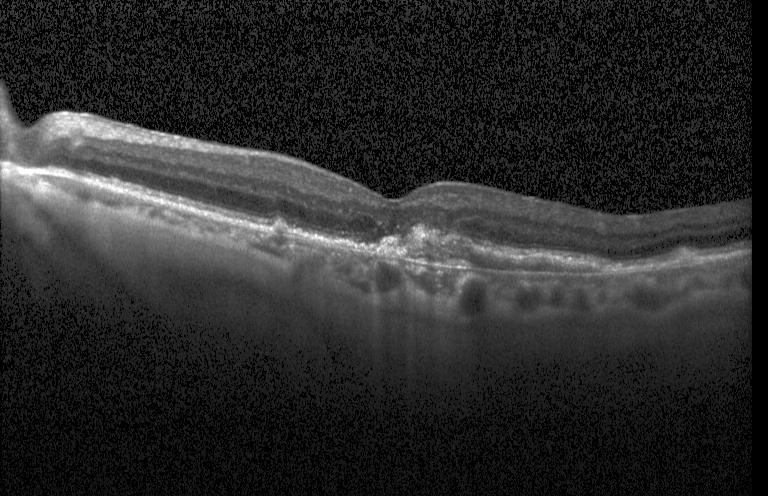

OCT line scan — Choroidal neovascularization.